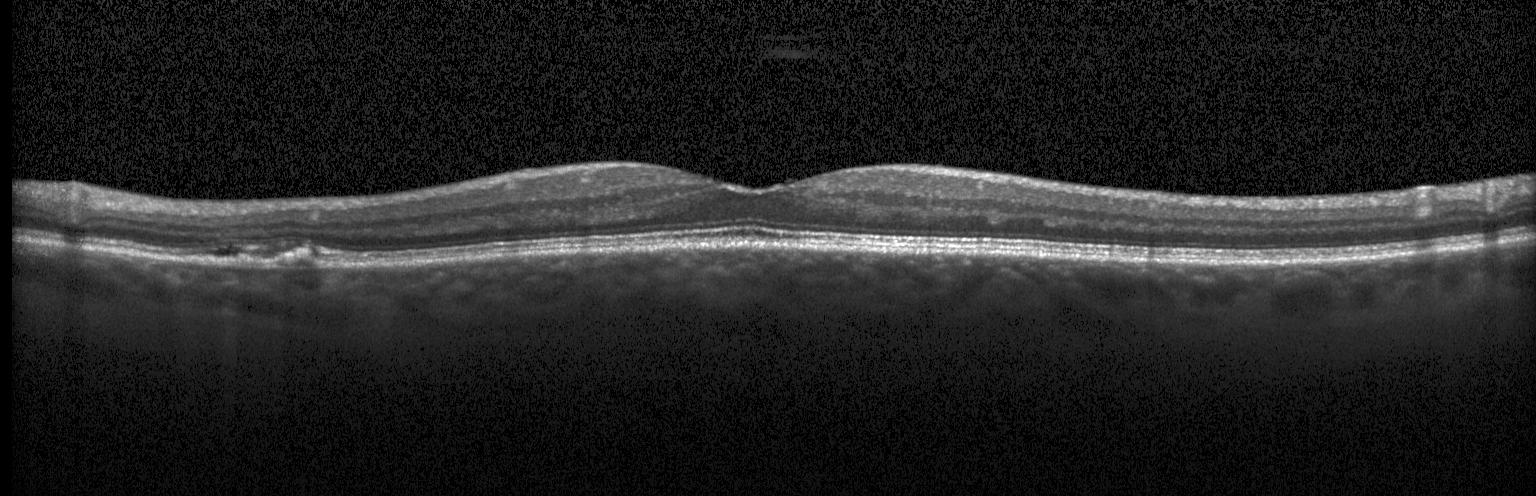
Finding: CNV.